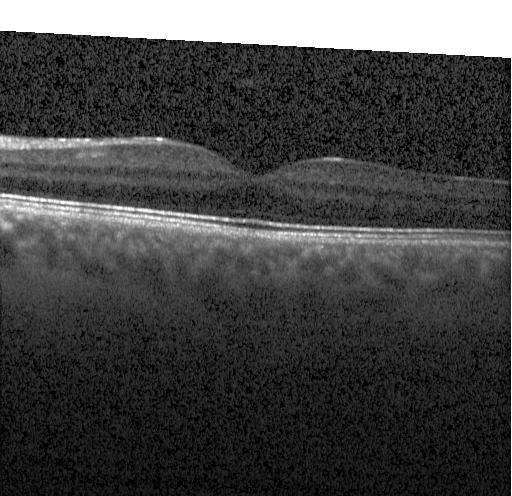

Heidelberg Spectralis OCT system · OCT B-scan — Diagnosis: no evidence of choroidal neovascularization, diabetic macular edema, or drusen.